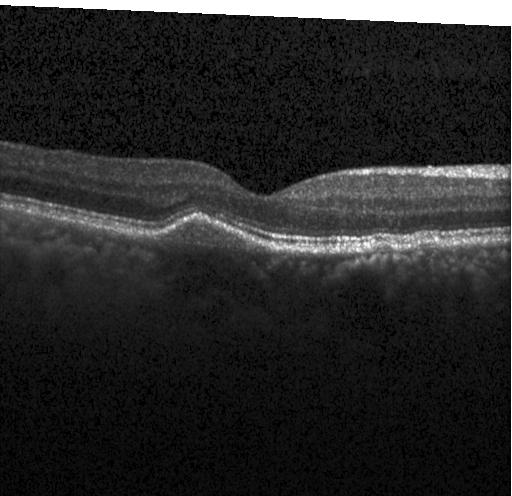 Optical coherence tomography B-scan — Diagnosis: sub-RPE drusenoid deposits.